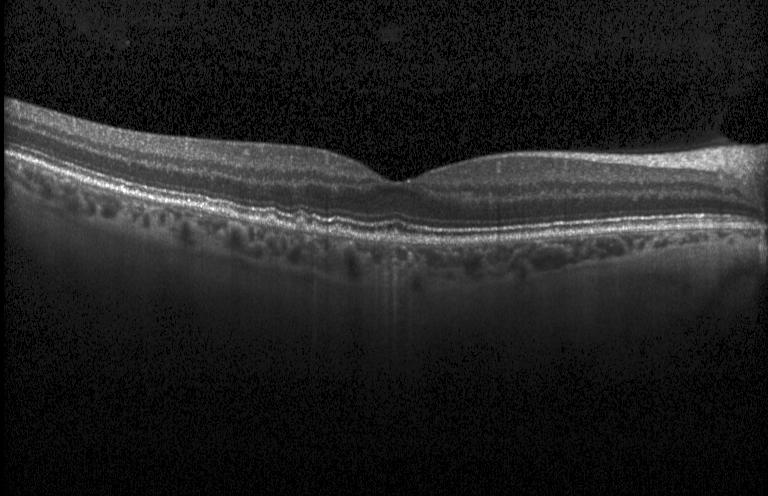 Diagnosis: multiple drusen.